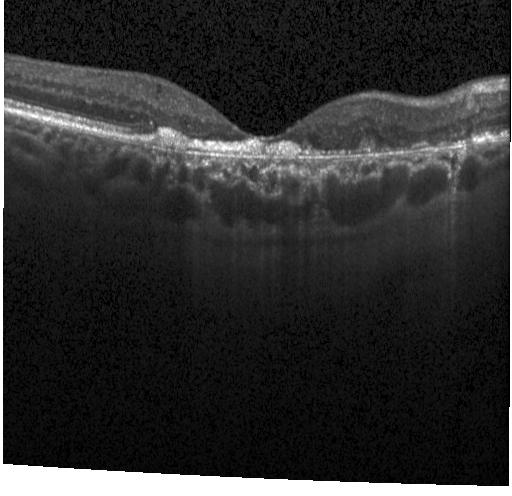

Acquired on a Heidelberg Spectralis · spectral-domain OCT · retinal OCT B-scan · horizontal scan through the fovea — Impression: a choroidal neovascular membrane.